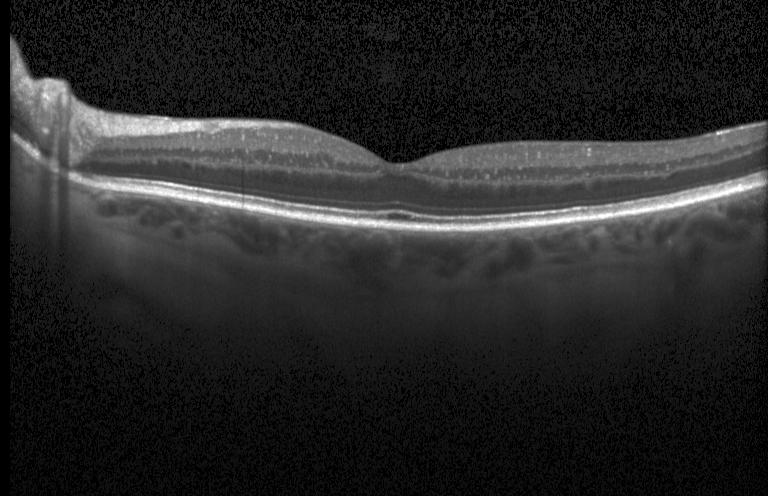

Diagnosis: no choroidal neovascularization, no diabetic macular edema, and no drusen.